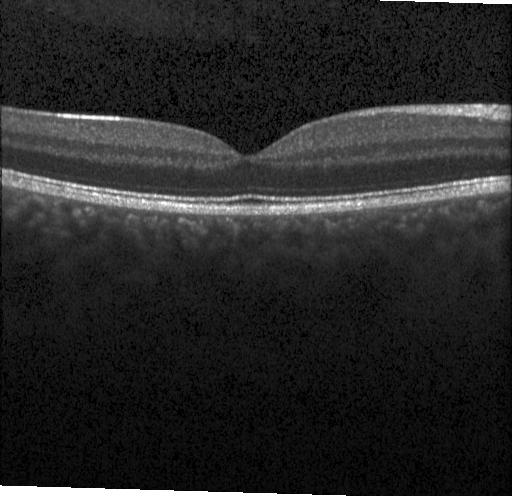

Fovea-centered, OCT line scan — Diagnosis: no evidence of CNV, DME, or drusen.